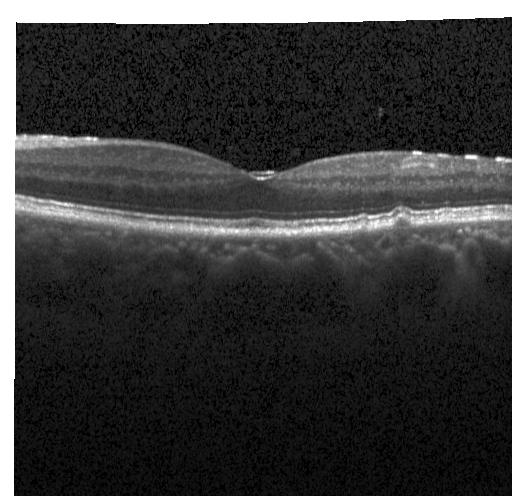
Macular scan; Heidelberg Spectralis OCT system; retinal OCT cross-section. Impression: drusen.